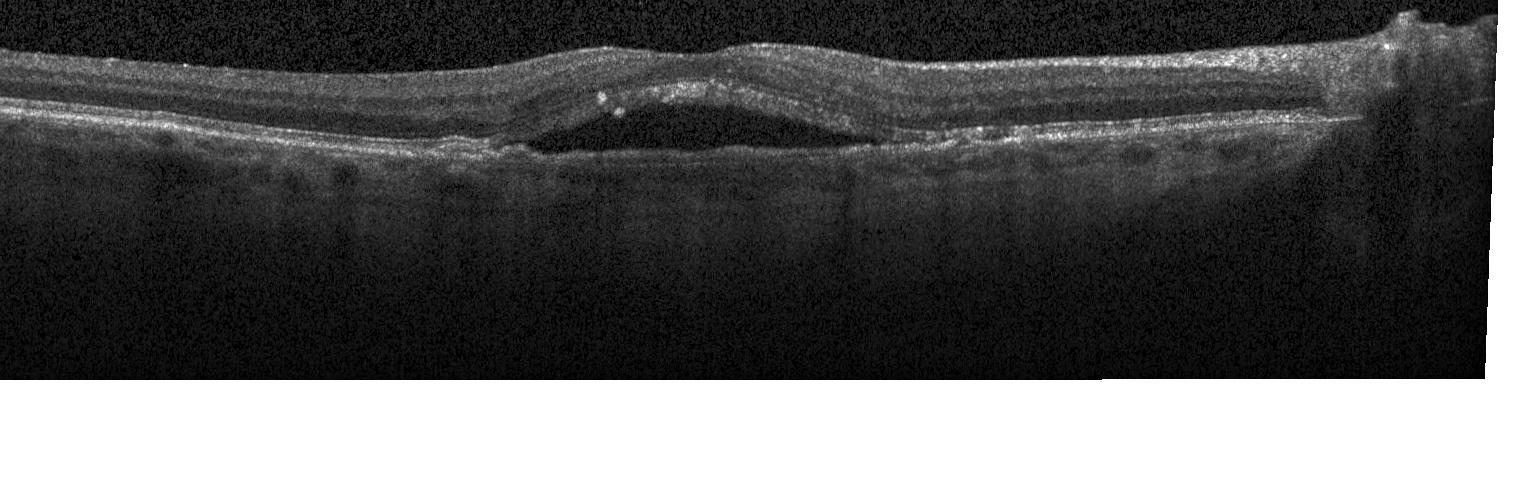 Finding: choroidal neovascularization (CNV).